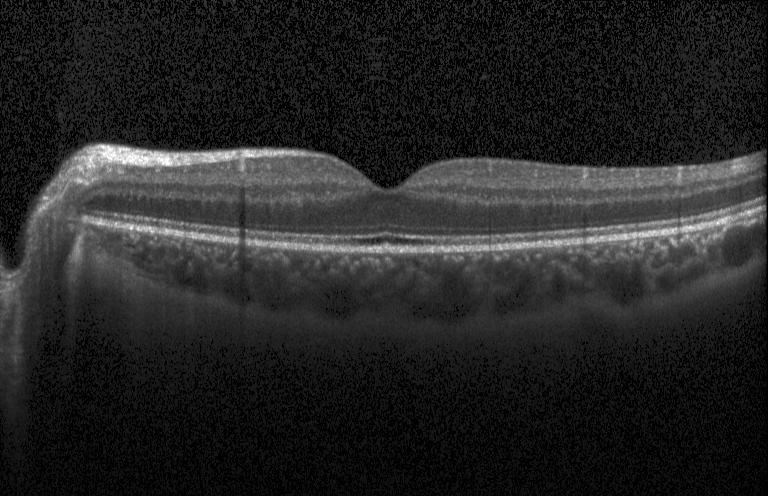
Fovea-centered. Spectral-domain OCT. Acquired on a Heidelberg Spectralis. OCT line scan. This B-scan demonstrates no choroidal neovascularization, diabetic macular edema, or drusen.